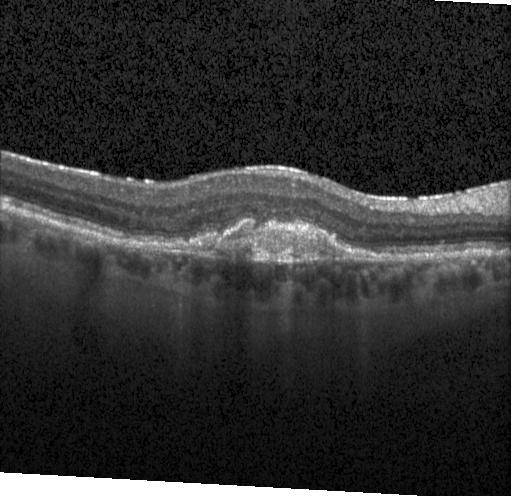

Macular OCT demonstrating CNV.